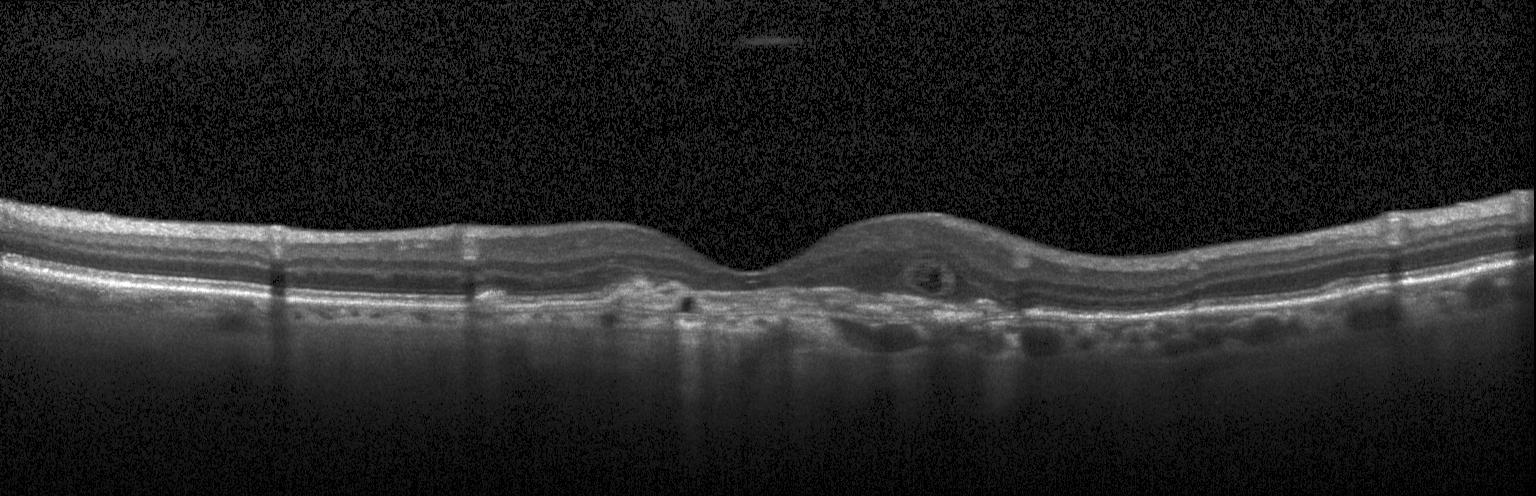 Macular scan, Heidelberg Spectralis OCT system, optical coherence tomography B-scan, spectral-domain optical coherence tomography
Dx: a choroidal neovascular membrane.